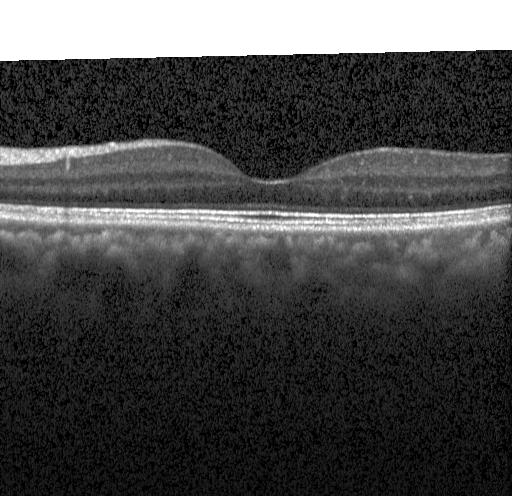 Retinal OCT cross-section, through the macula, instrument: Heidelberg Spectralis — Impression: no choroidal neovascularization, no diabetic macular edema, and no drusen.